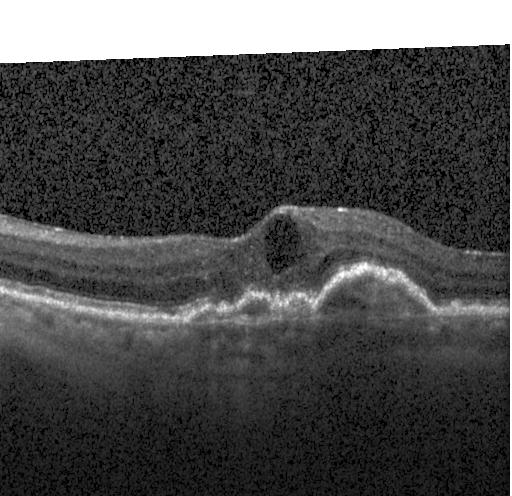 Horizontal scan through the fovea. Acquired on a Heidelberg Spectralis. Retinal OCT cross-section. SD-OCT — Diagnosis: choroidal neovascularization.